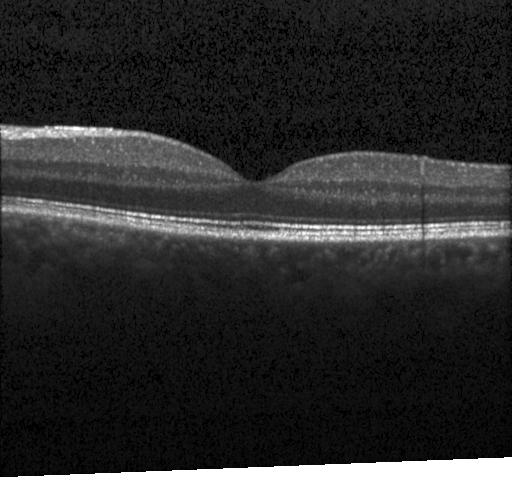
Retinal OCT B-scan.
This B-scan demonstrates neither choroidal neovascularization, diabetic macular edema, nor drusen.